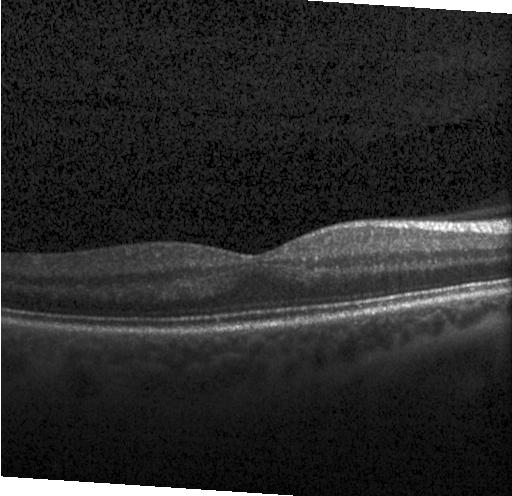 Dx: no CNV, DME, or drusen.